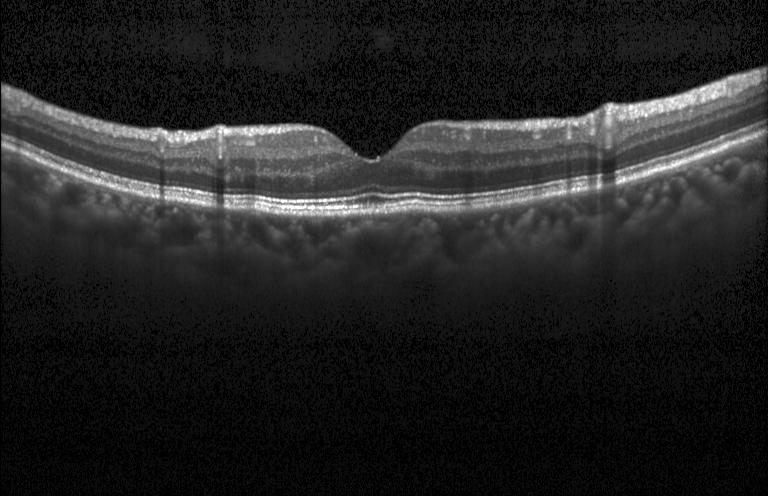
The scan shows no evidence of CNV, DME, or drusen.